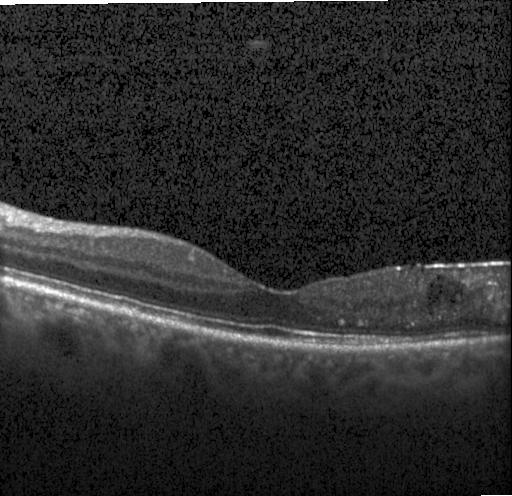 Spectral-domain OCT, acquired on a Heidelberg Spectralis, optical coherence tomography B-scan. OCT finding: diabetic macular edema (DME).